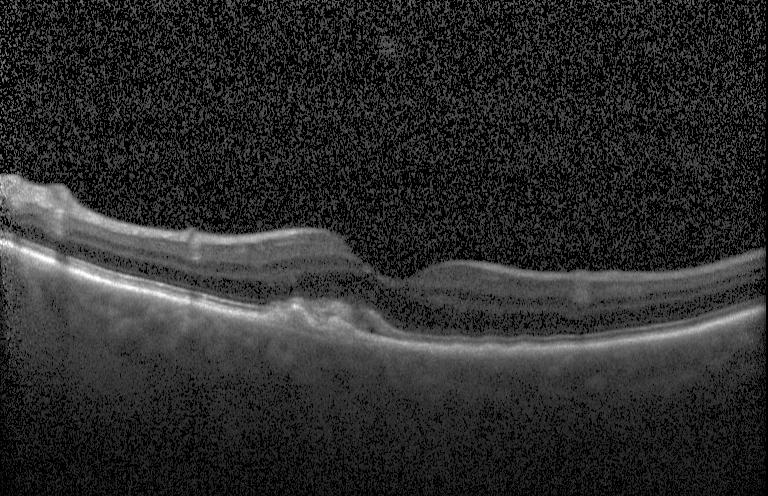

Retinal OCT B-scan, spectral-domain OCT, Heidelberg Spectralis OCT system.
Diagnosis: choroidal neovascularization.